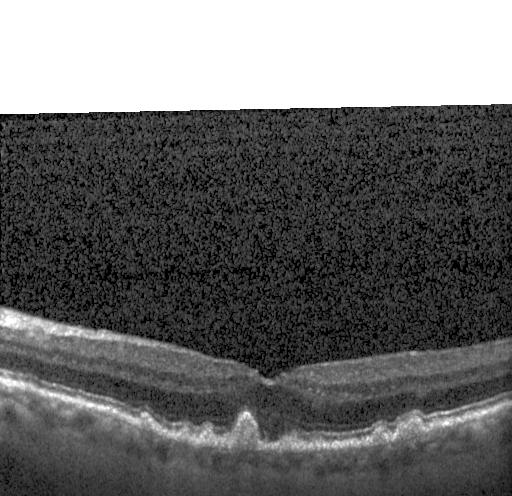 Finding: sub-RPE drusenoid deposits.